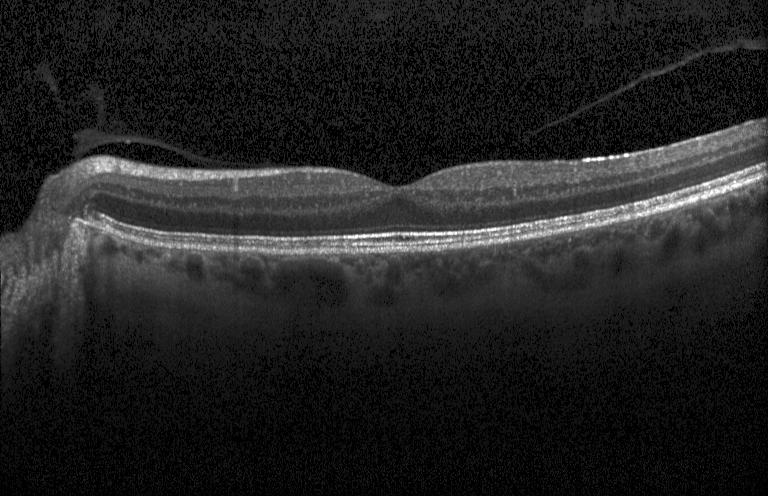
Spectral-domain optical coherence tomography · retinal OCT cross-section
Diagnosis: no CNV, DME, or drusen.